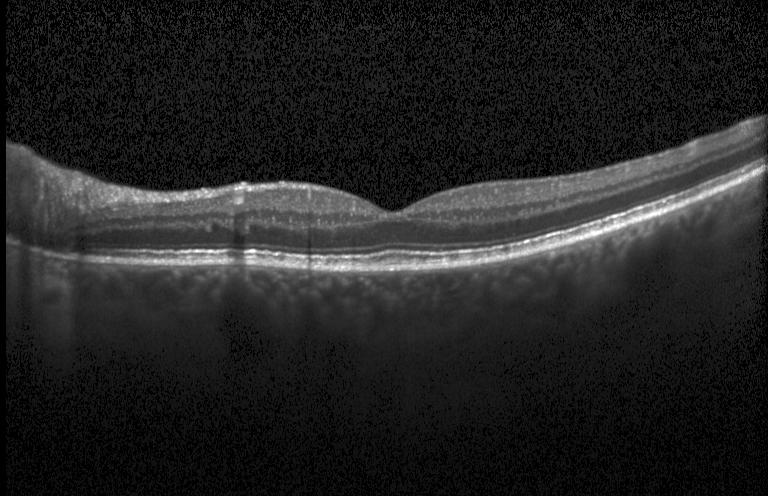
Fovea-centered, Heidelberg Spectralis, optical coherence tomography scan, spectral-domain optical coherence tomography. Neither choroidal neovascularization, diabetic macular edema, nor drusen.